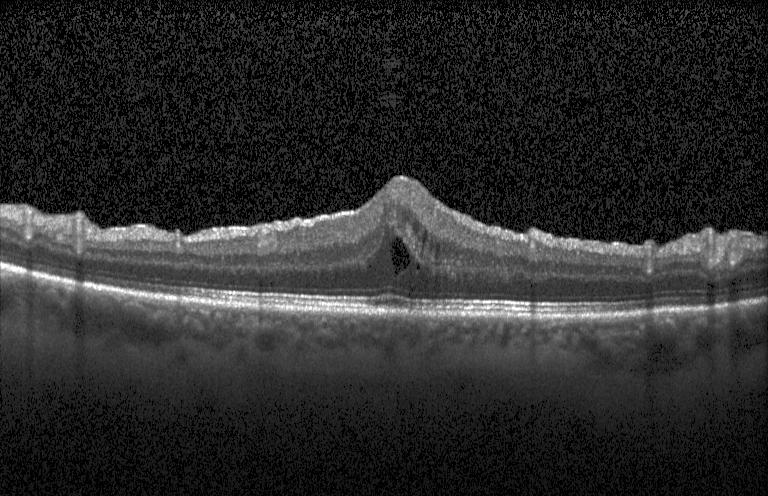
Retinal OCT cross-section
Finding: diabetic macular edema.